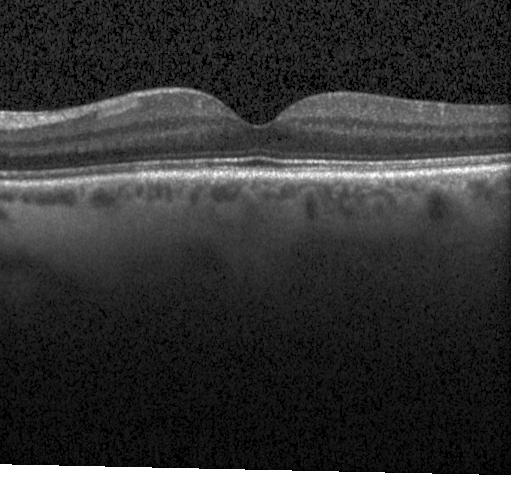 Optical coherence tomography B-scan, SD-OCT, Heidelberg Spectralis, macular scan — Diagnosis: no CNV, no DME, and no drusen.